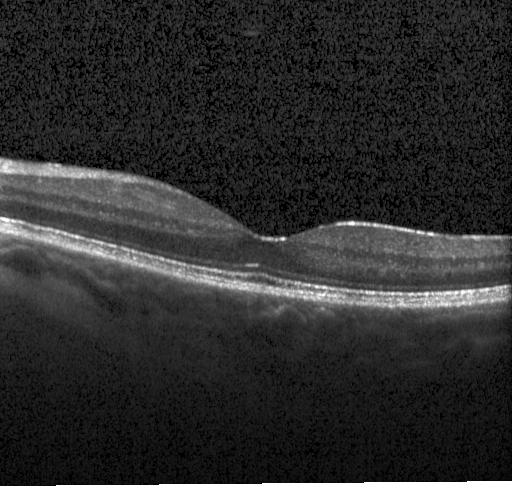

Impression: no CNV, no DME, and no drusen.